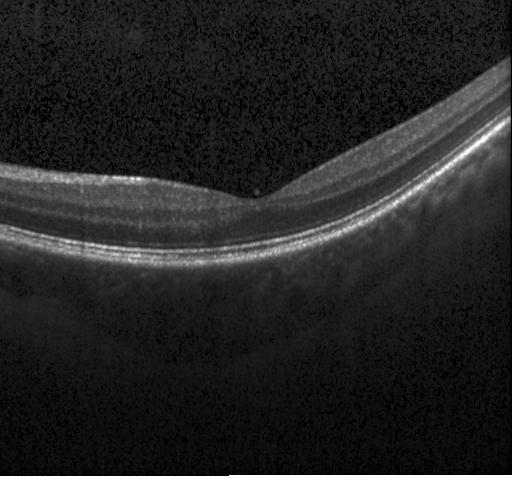 Heidelberg Spectralis, optical coherence tomography scan. Assessment: no choroidal neovascularization, diabetic macular edema, or drusen.